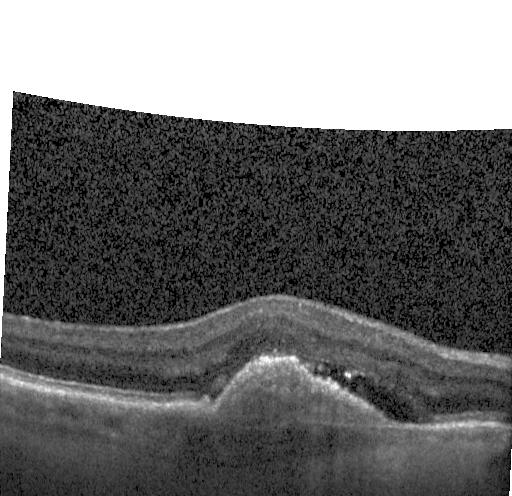 Fovea-centered · optical coherence tomography scan — CNV.